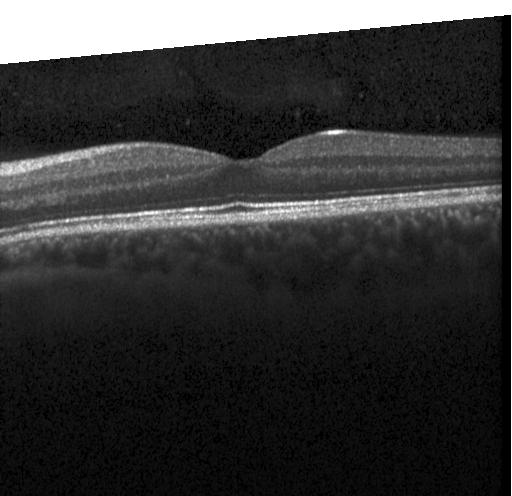

OCT B-scan — Impression: no evidence of choroidal neovascularization, diabetic macular edema, or drusen.